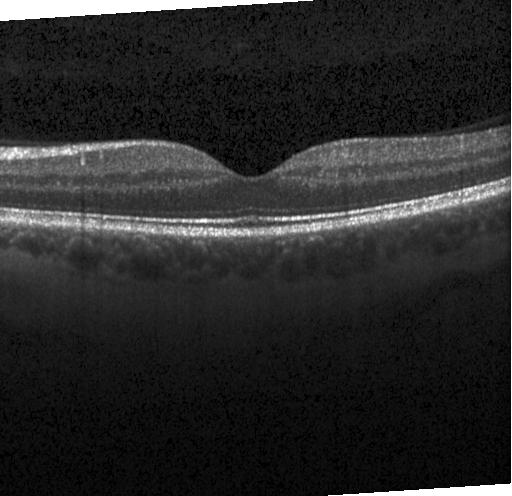
Retinal OCT cross-section showing no choroidal neovascularization, diabetic macular edema, or drusen.